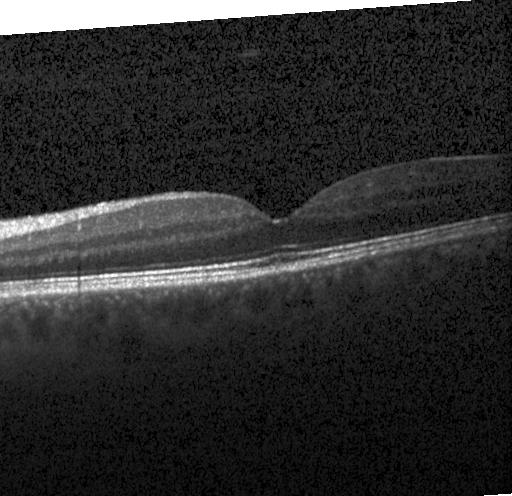
Macular OCT demonstrating neither choroidal neovascularization, diabetic macular edema, nor drusen.